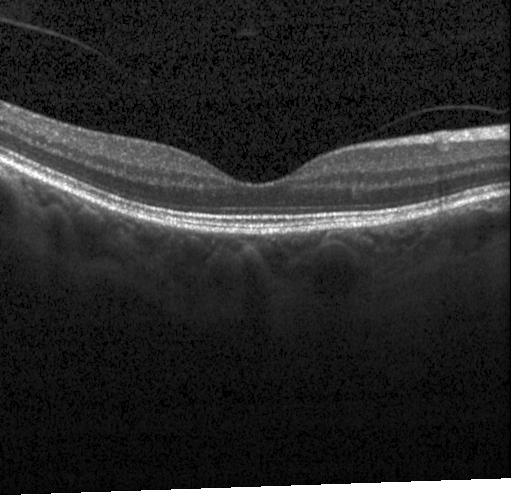 Macular OCT: no CNV, DME, or drusen.